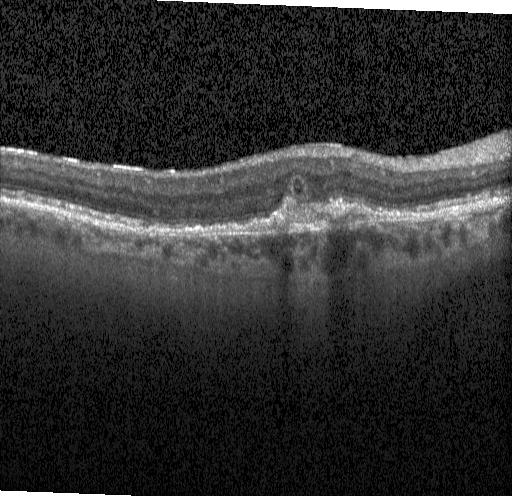

OCT B-scan
Macular OCT: a choroidal neovascular membrane.